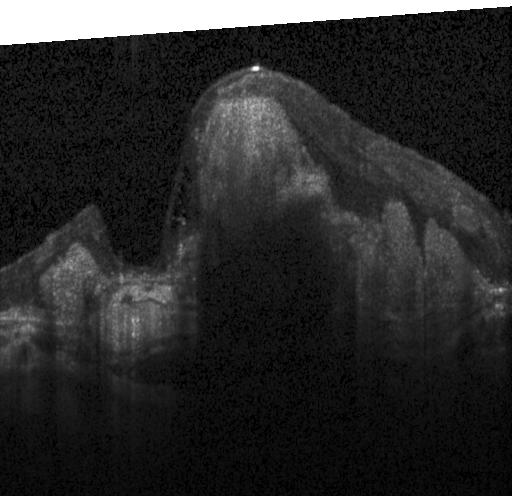 Instrument: Heidelberg Spectralis. Spectral-domain OCT. Through the macula. Optical coherence tomography B-scan. OCT finding: a choroidal neovascular membrane.